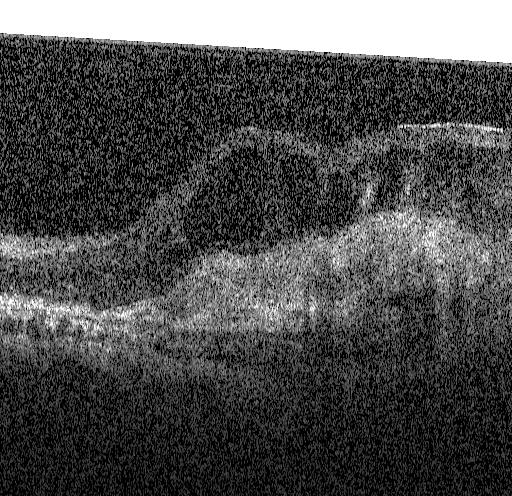 Retinal OCT B-scan. Spectral-domain optical coherence tomography
Finding: choroidal neovascularization.